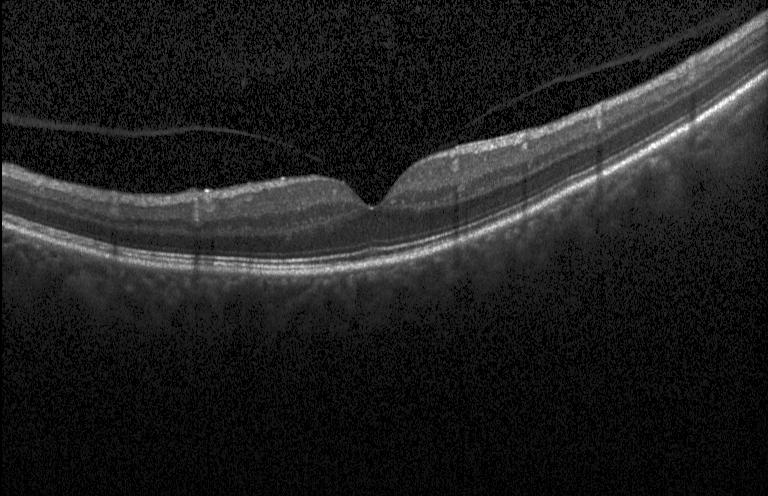
Heidelberg Spectralis. Fovea-centered. Optical coherence tomography B-scan — Finding: no evidence of choroidal neovascularization, diabetic macular edema, or drusen.